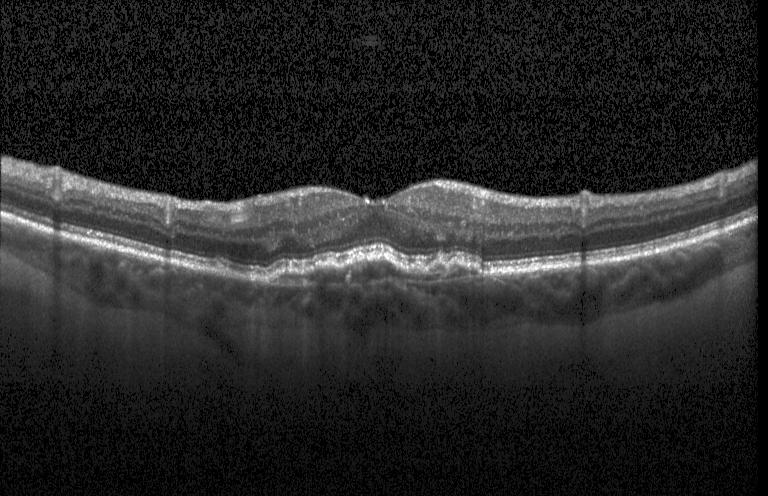

OCT B-scan; fovea-centered — Diagnosis: choroidal neovascularization (CNV).